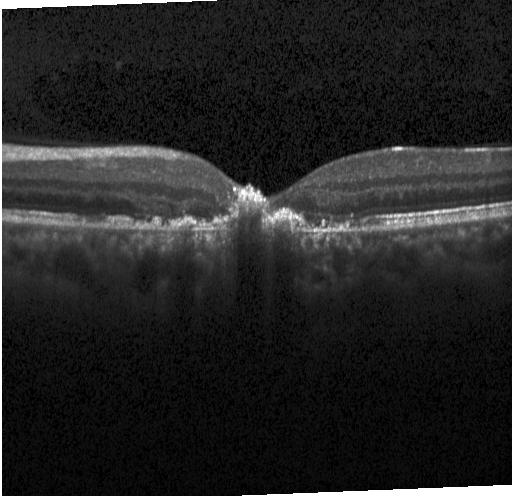

Spectral-domain OCT. Retinal OCT B-scan. Heidelberg Spectralis. Macular scan. Diagnosis: choroidal neovascularization.